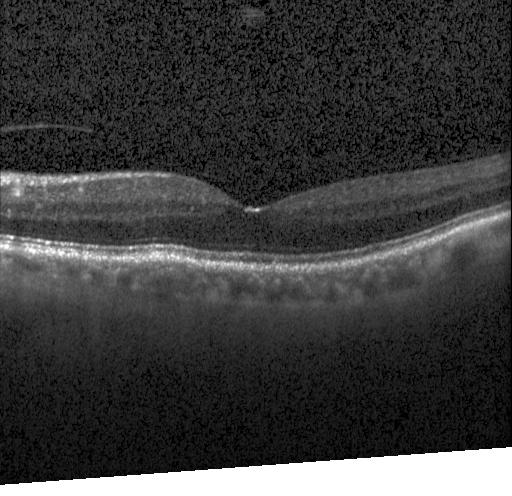 Impression: no choroidal neovascularization, diabetic macular edema, or drusen.